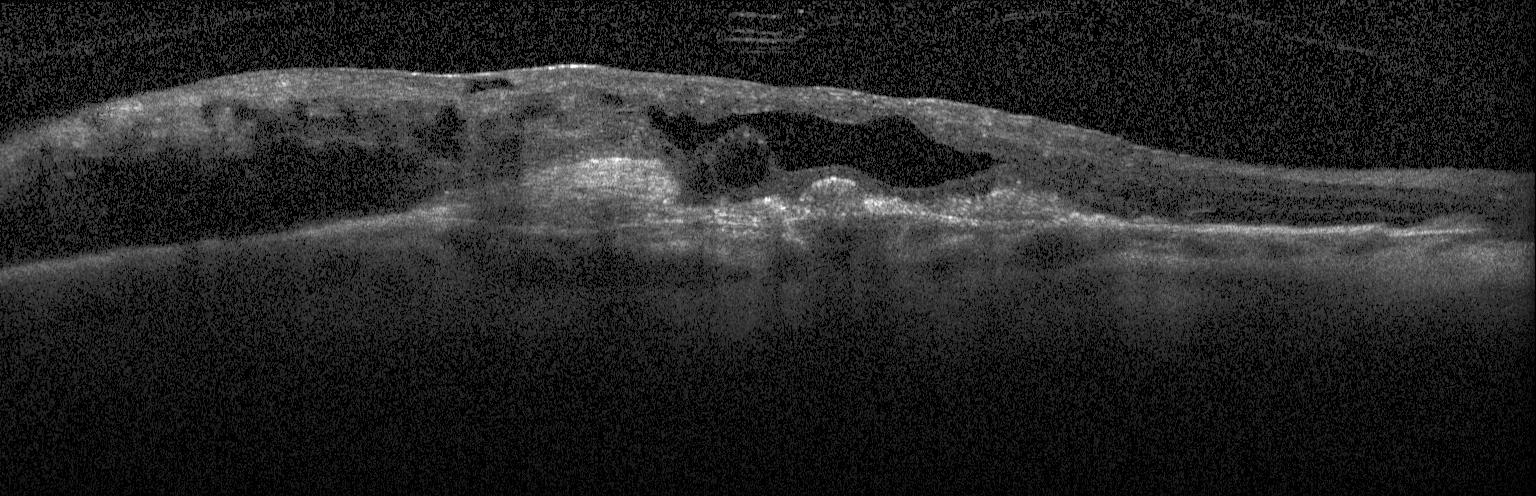

Retinal OCT cross-section, macular scan, Heidelberg Spectralis, spectral-domain OCT.
The scan shows a choroidal neovascular membrane.